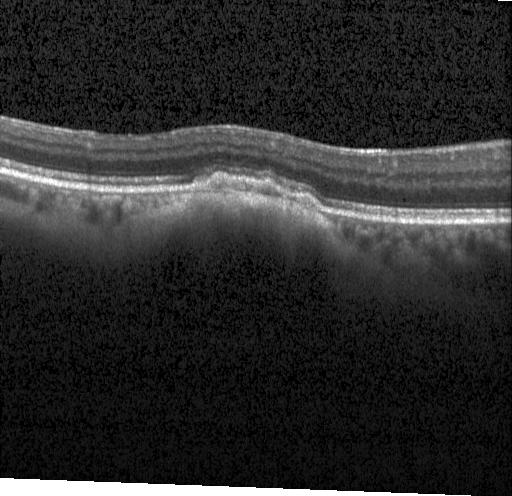
Heidelberg Spectralis, retinal OCT B-scan
Impression: choroidal neovascularization (CNV).